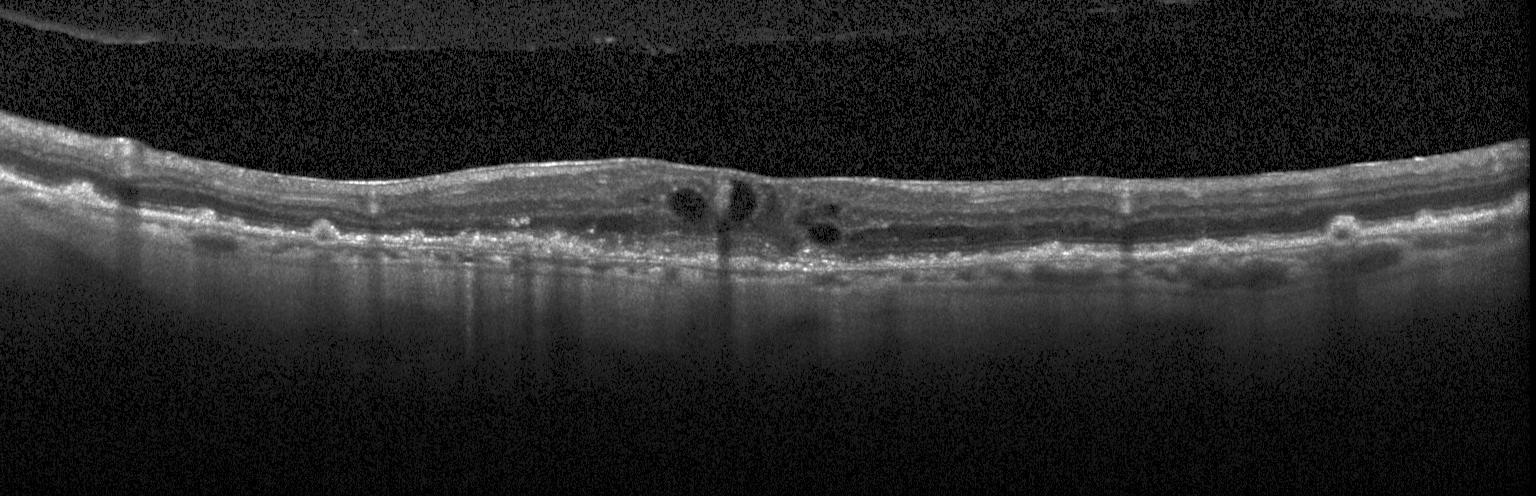 Finding: CNV.